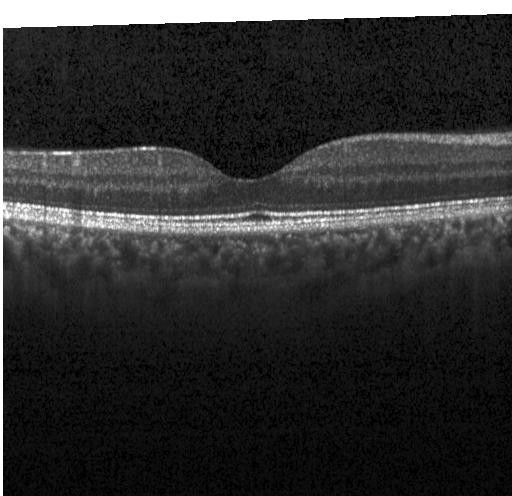

Acquired on a Heidelberg Spectralis; OCT B-scan. Finding: no evidence of choroidal neovascularization, diabetic macular edema, or drusen.